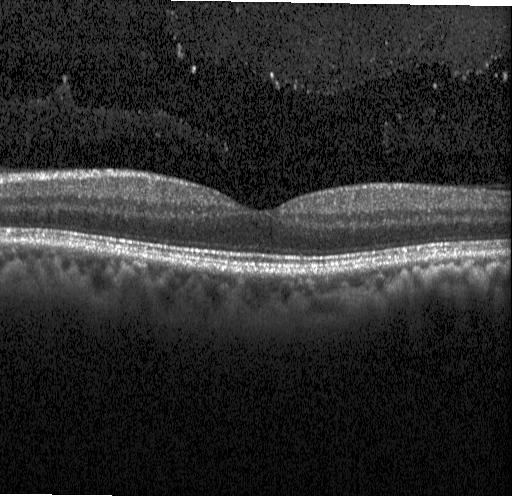
Diagnosis: neither choroidal neovascularization, diabetic macular edema, nor drusen.